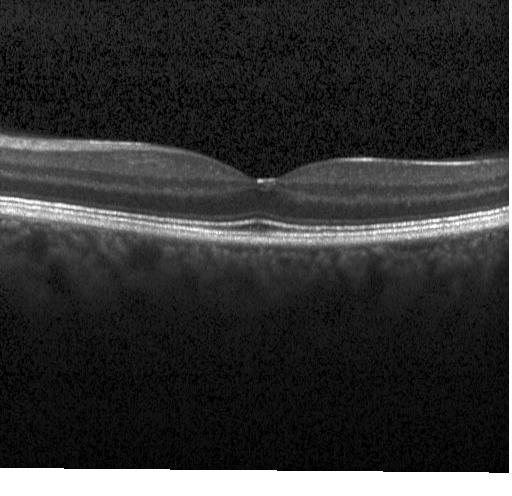
Optical coherence tomography B-scan. The scan shows no choroidal neovascularization, diabetic macular edema, or drusen.